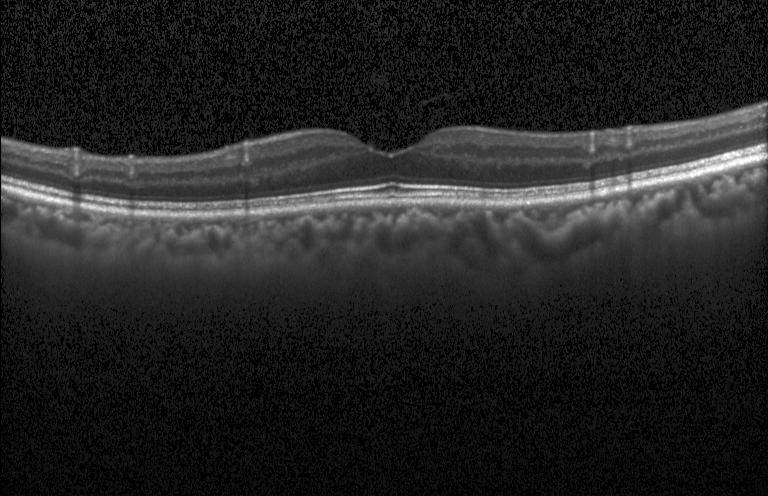

OCT scan showing neither choroidal neovascularization, diabetic macular edema, nor drusen.